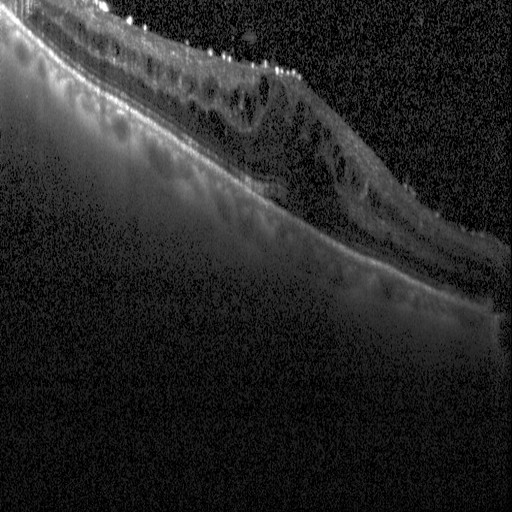 Optical coherence tomography B-scan — Dx: DME.